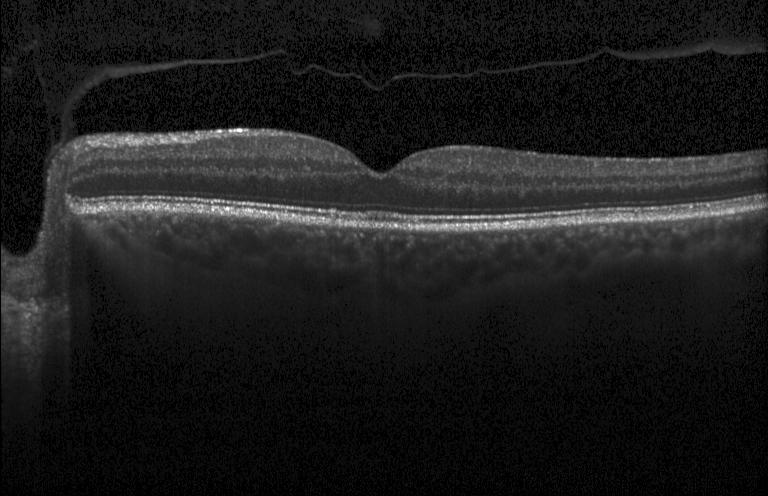 Retinal OCT B-scan.
No evidence of choroidal neovascularization, diabetic macular edema, or drusen.